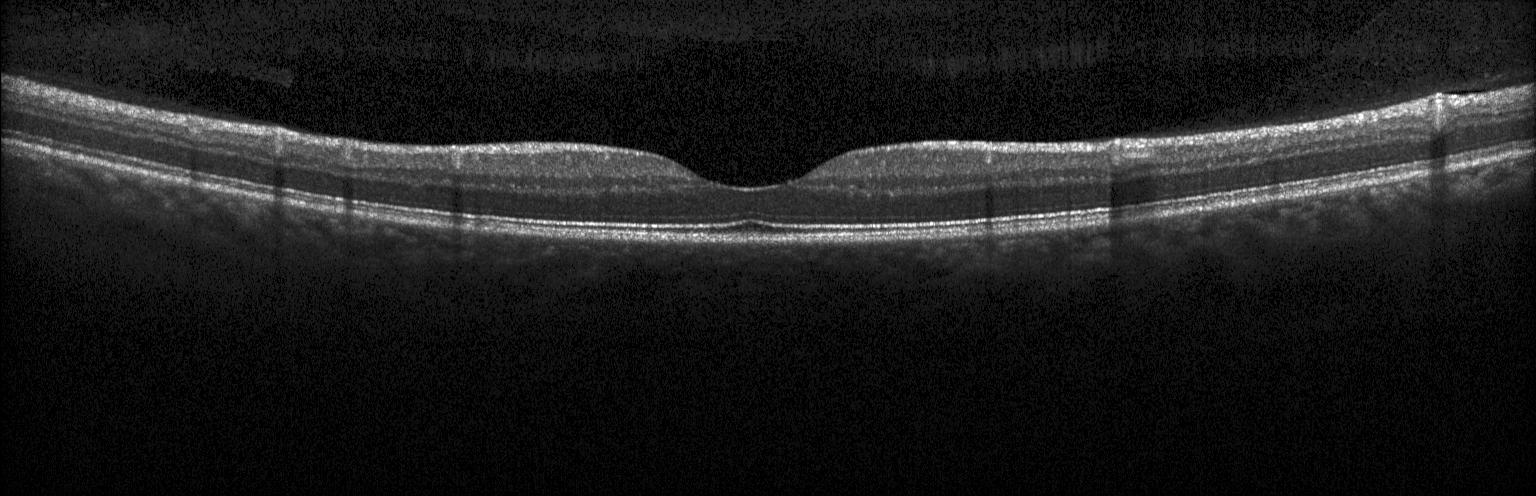

Centered on the fovea, optical coherence tomography scan.
OCT finding: no choroidal neovascularization, no diabetic macular edema, and no drusen.